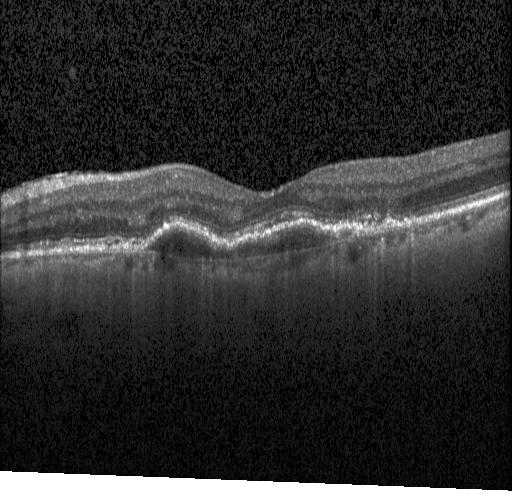

Retinal OCT cross-section · centered on the fovea · spectral-domain optical coherence tomography.
The scan shows a choroidal neovascular membrane.